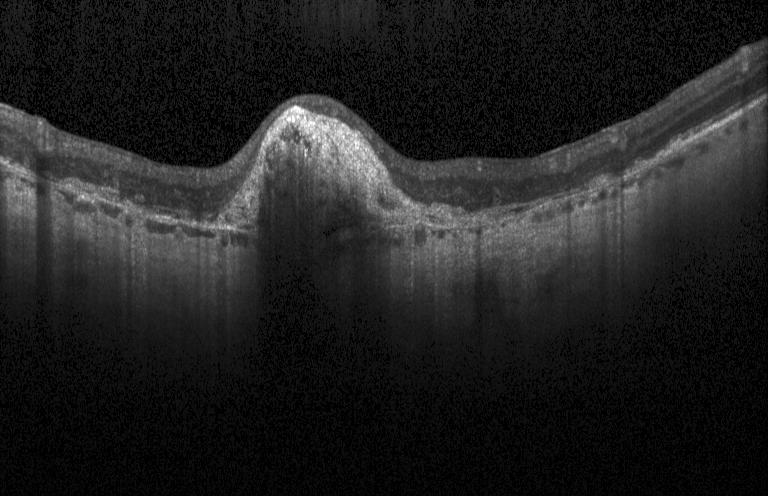

Fovea-centered. Spectral-domain optical coherence tomography. Instrument: Heidelberg Spectralis. Optical coherence tomography scan
Finding: a choroidal neovascular membrane.